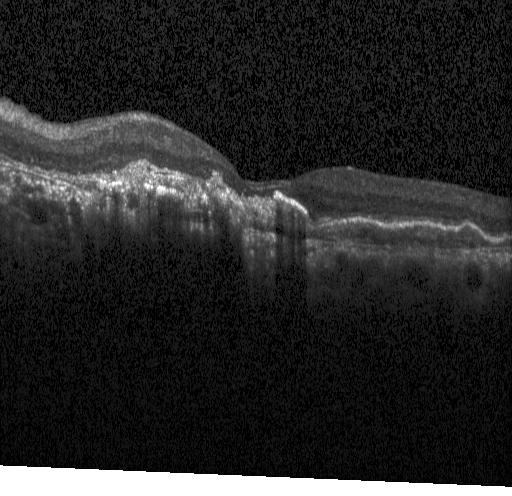
The scan shows a choroidal neovascular membrane.